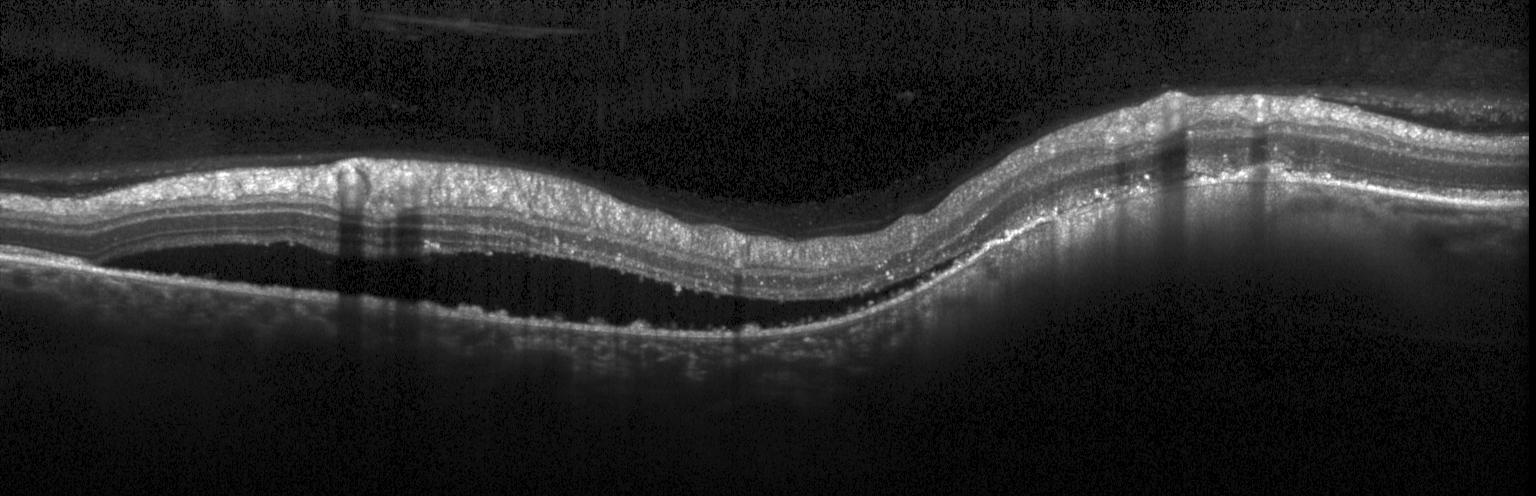

The scan shows choroidal neovascularization.